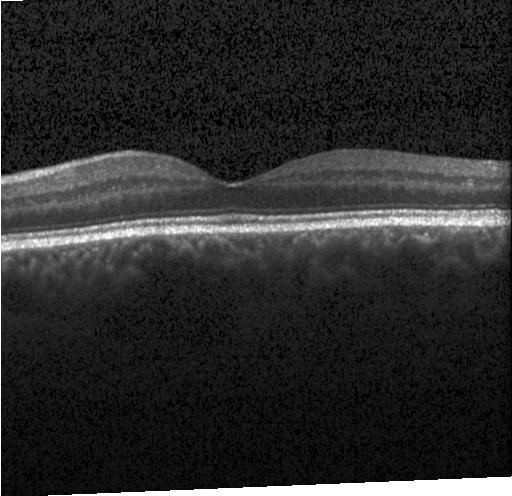 Dx: no CNV, no DME, and no drusen.